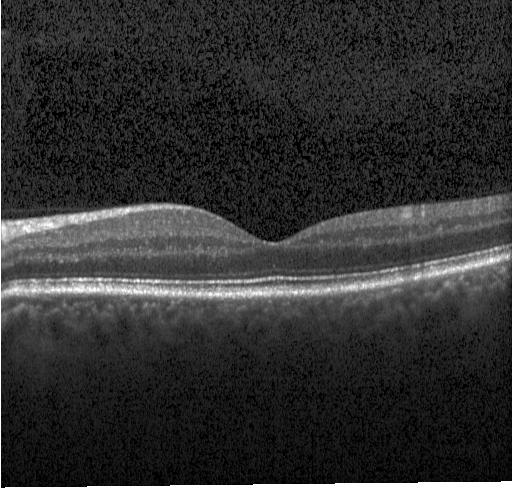 Assessment: no evidence of choroidal neovascularization, diabetic macular edema, or drusen.